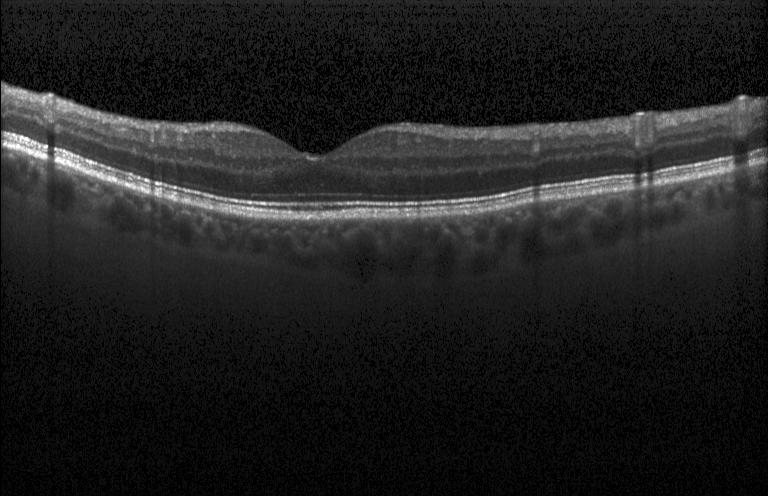
Finding: no CNV, no DME, and no drusen.